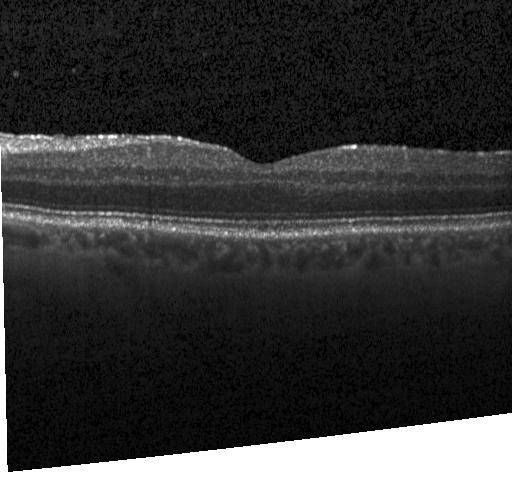 Through the macula; acquired on a Heidelberg Spectralis; retinal OCT cross-section. Finding: no choroidal neovascularization, diabetic macular edema, or drusen.